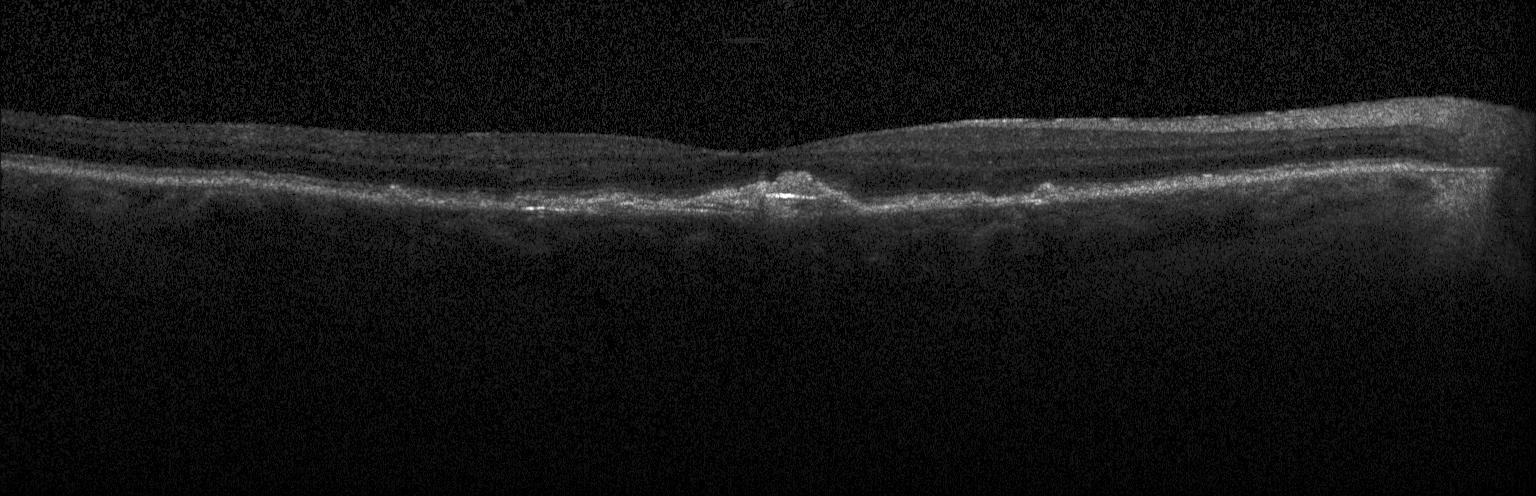

Heidelberg Spectralis. OCT line scan. Spectral-domain optical coherence tomography — A choroidal neovascular membrane.